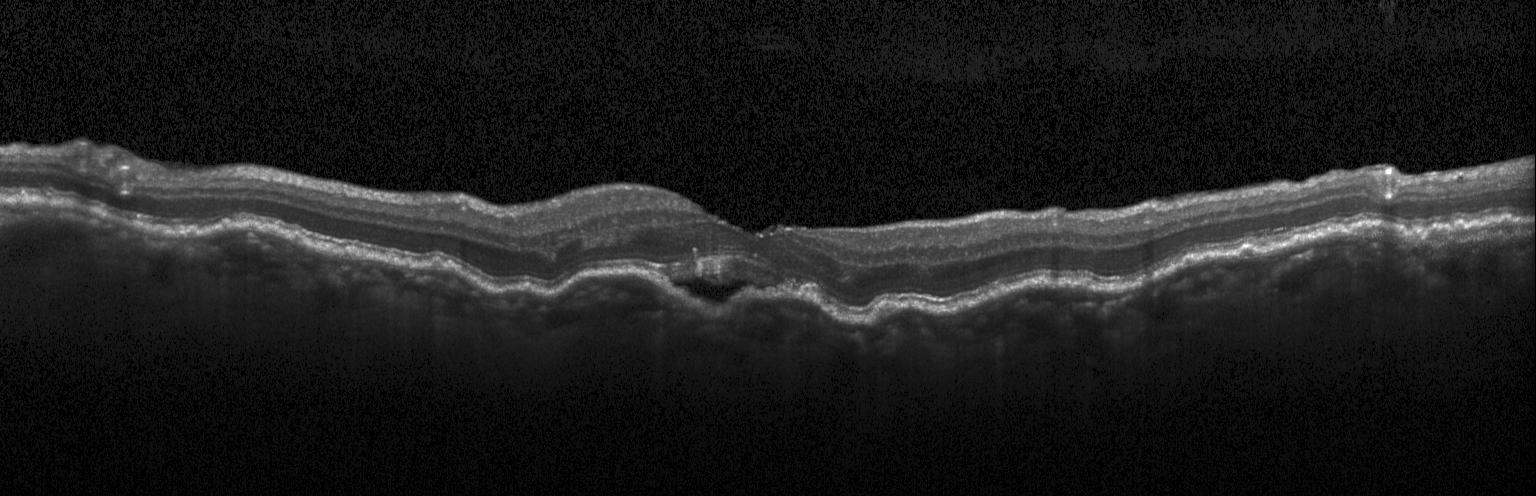
OCT B-scan showing choroidal neovascularization.